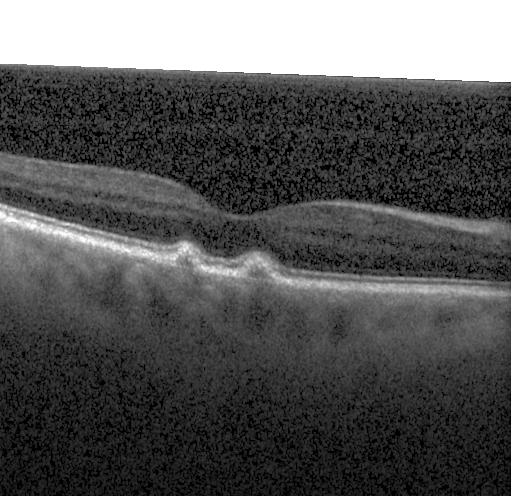
Spectral-domain OCT · centered on the fovea · OCT line scan. OCT finding: sub-RPE drusenoid deposits.